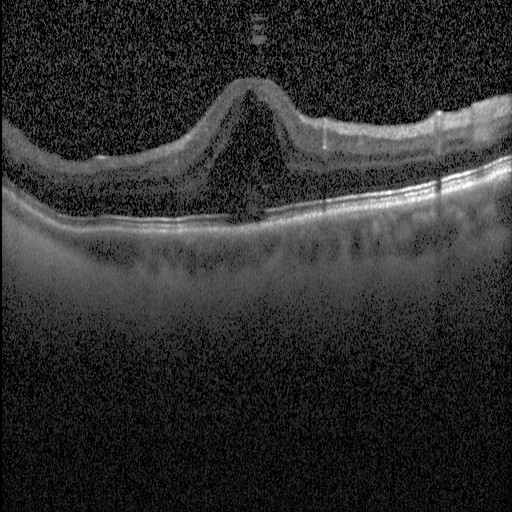

Spectral-domain OCT B-scan: diabetic macular edema (DME).